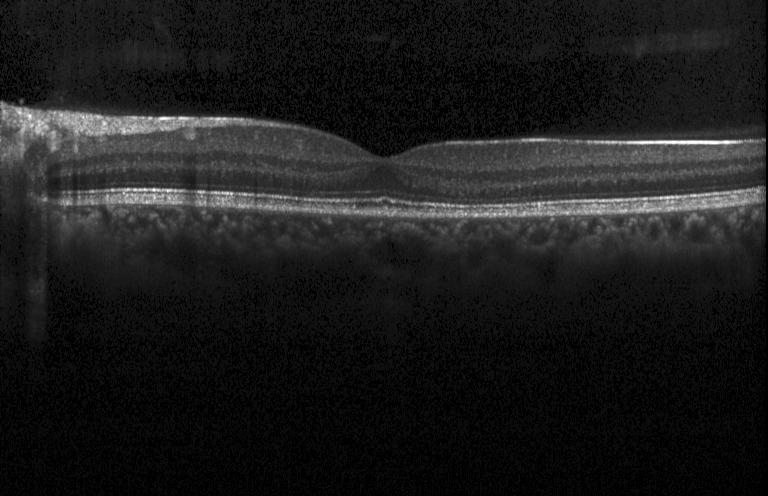 Macular scan. OCT B-scan.
Impression: no CNV, no DME, and no drusen.